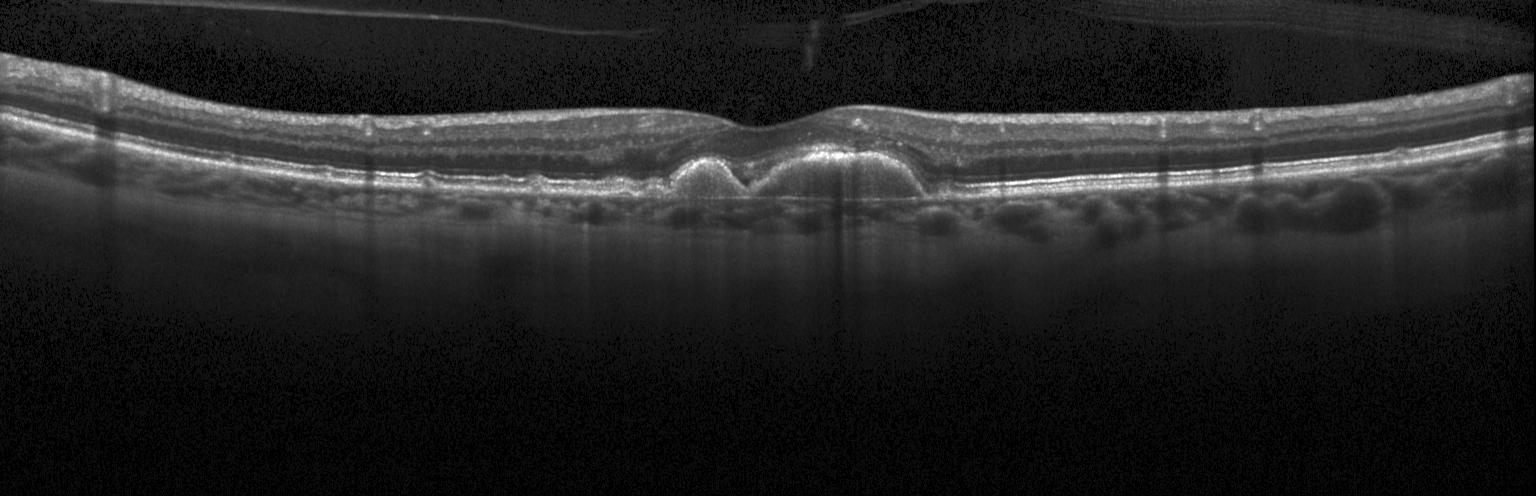
Impression: a choroidal neovascular membrane.